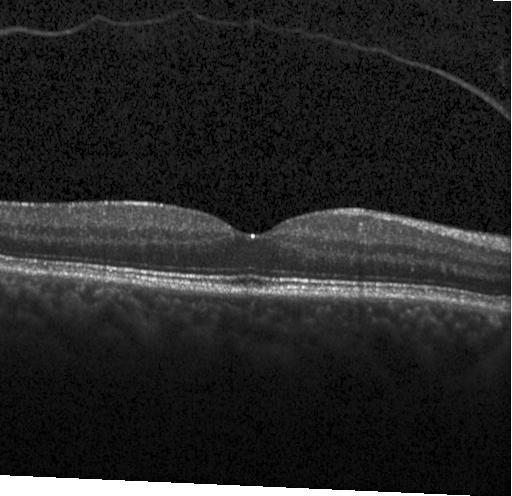 Optical coherence tomography B-scan. Finding: no evidence of choroidal neovascularization, diabetic macular edema, or drusen.